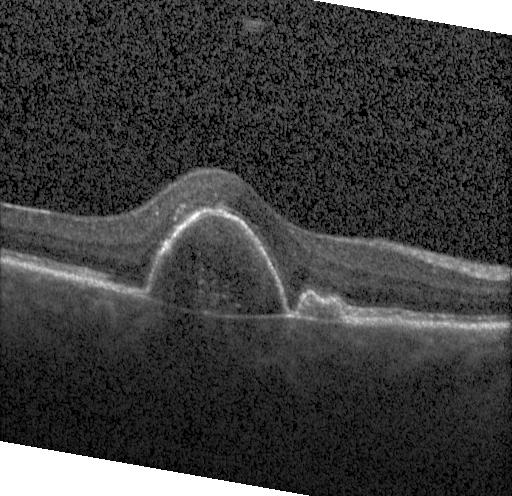
Heidelberg Spectralis. Centered on the fovea. OCT B-scan. Spectral-domain OCT.
Impression: CNV.